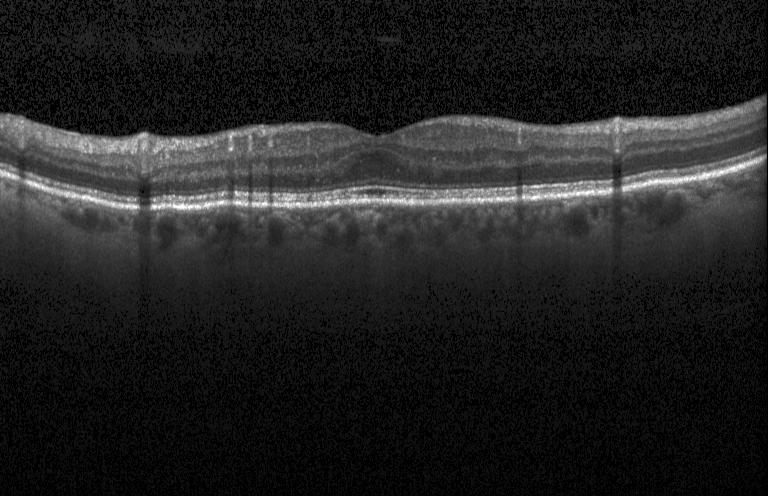
Retinal OCT B-scan — Finding: no choroidal neovascularization, no diabetic macular edema, and no drusen.